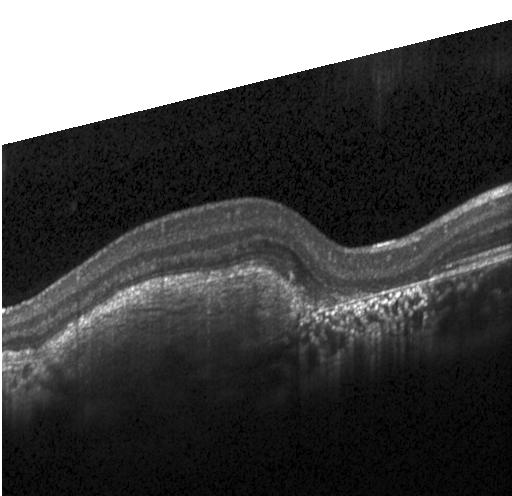

Diagnosis: choroidal neovascularization.